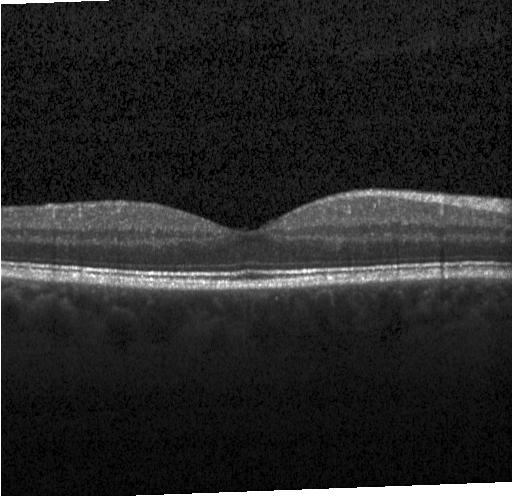

Heidelberg Spectralis; retinal OCT cross-section; spectral-domain optical coherence tomography; macular scan
Diagnosis: no CNV, DME, or drusen.